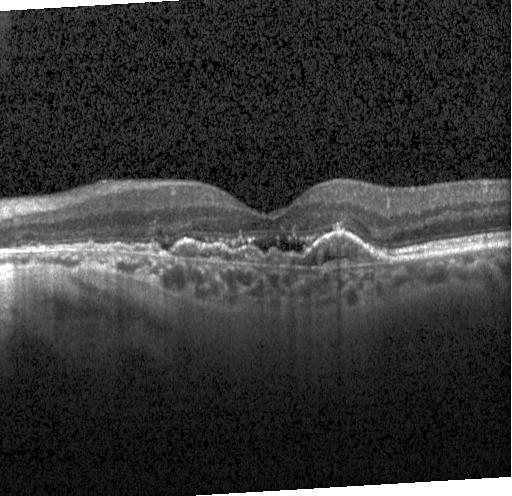
Horizontal scan through the fovea. OCT B-scan. Impression: a choroidal neovascular membrane.